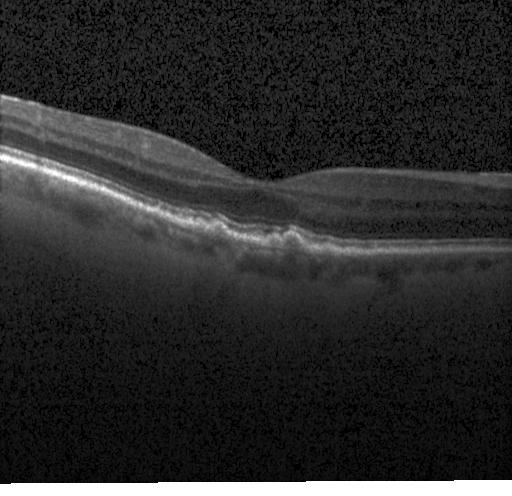 Instrument: Heidelberg Spectralis. Optical coherence tomography B-scan.
Assessment: multiple drusen.